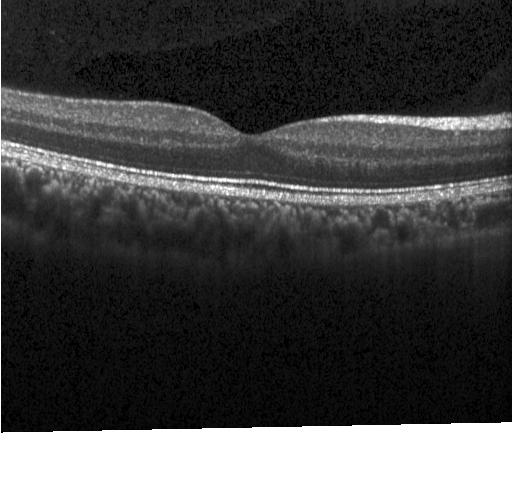

SD-OCT; centered on the fovea; OCT line scan.
This B-scan demonstrates no evidence of CNV, DME, or drusen.